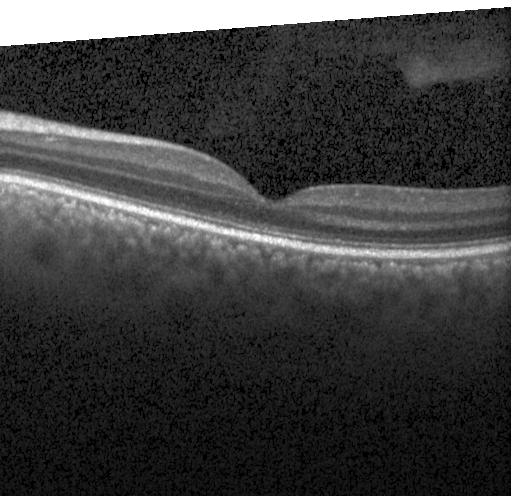 Fovea-centered; optical coherence tomography B-scan. Assessment: neither choroidal neovascularization, diabetic macular edema, nor drusen.